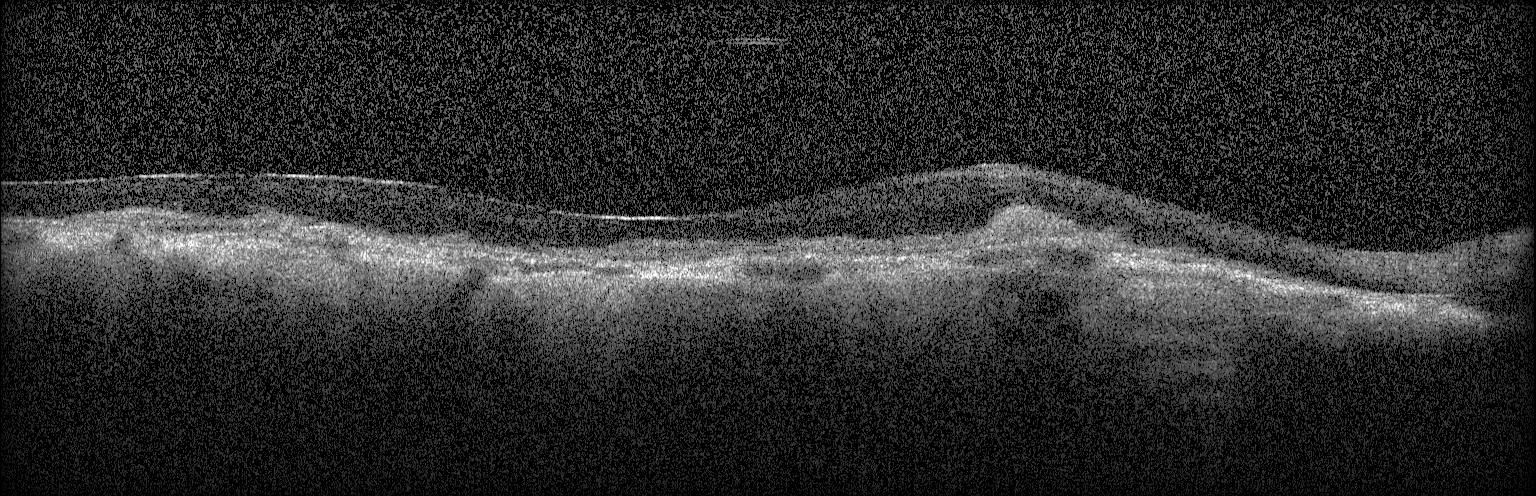

Impression: CNV.